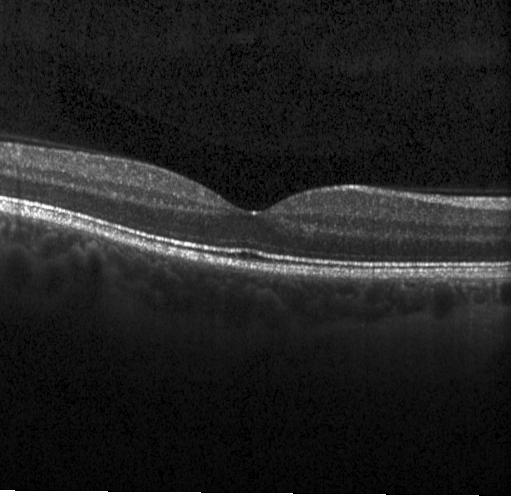
The scan shows no choroidal neovascularization, no diabetic macular edema, and no drusen.